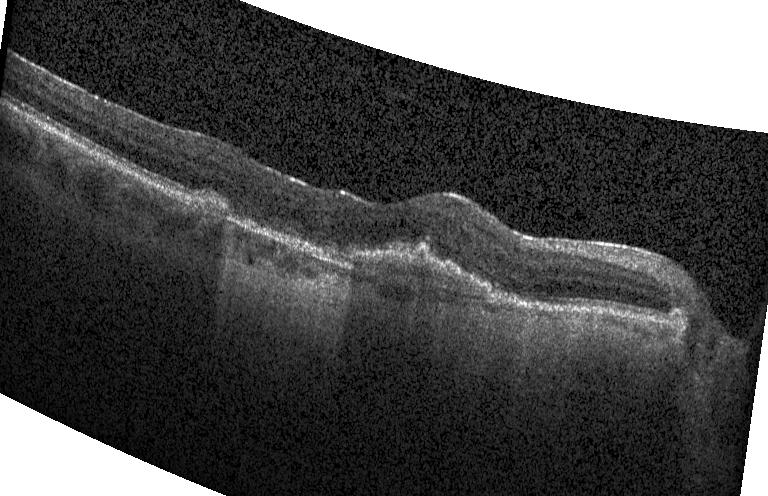
Fovea-centered; Heidelberg Spectralis; retinal OCT cross-section — Dx: a choroidal neovascular membrane.